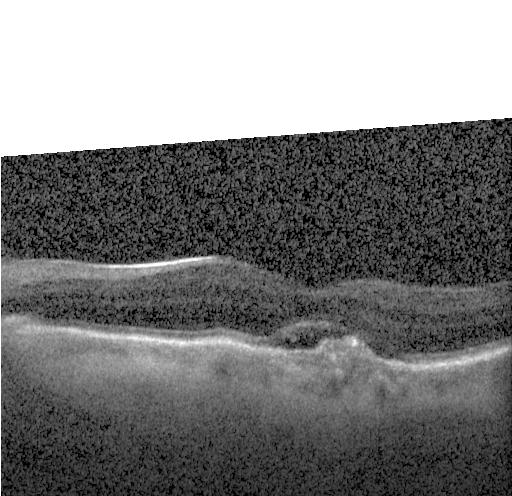
Instrument: Heidelberg Spectralis. Retinal OCT cross-section. Through the macula. A choroidal neovascular membrane.